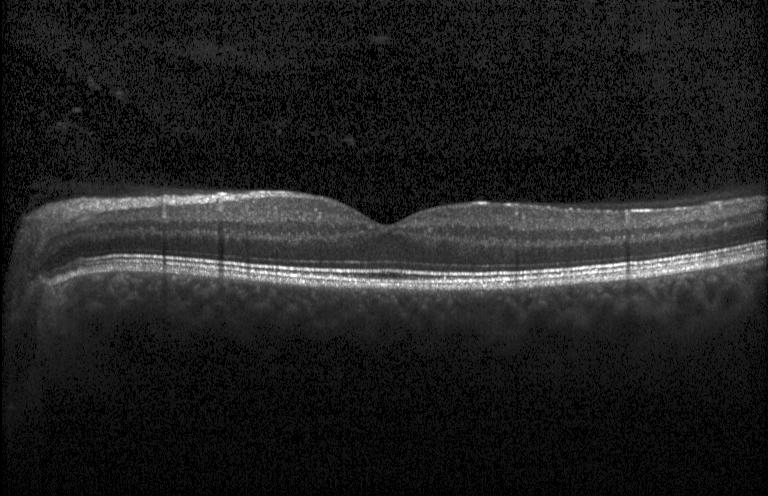 Diagnosis: no choroidal neovascularization, no diabetic macular edema, and no drusen.